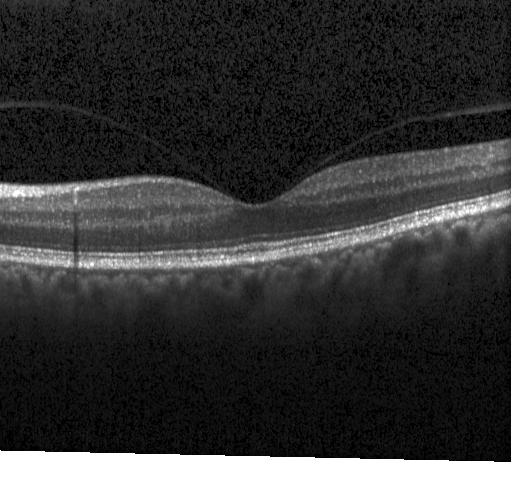 Macular OCT demonstrating no choroidal neovascularization, no diabetic macular edema, and no drusen.